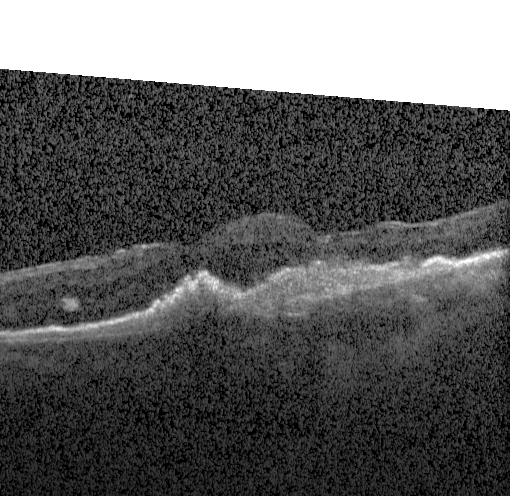
Dx: a choroidal neovascular membrane.